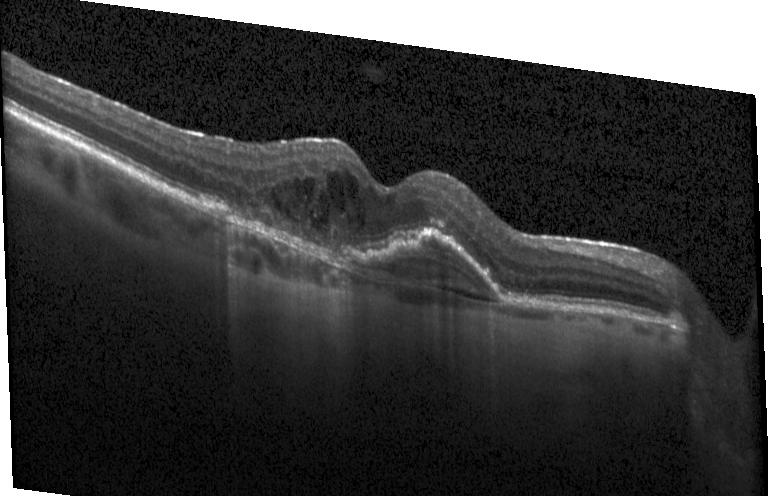
Heidelberg Spectralis OCT system, retinal OCT cross-section, spectral-domain optical coherence tomography.
Finding: choroidal neovascularization (CNV).